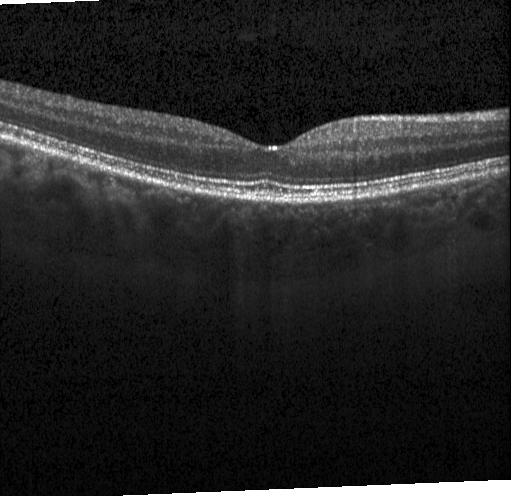 Heidelberg Spectralis. Centered on the fovea. Retinal OCT B-scan. Spectral-domain OCT.
No CNV, DME, or drusen.